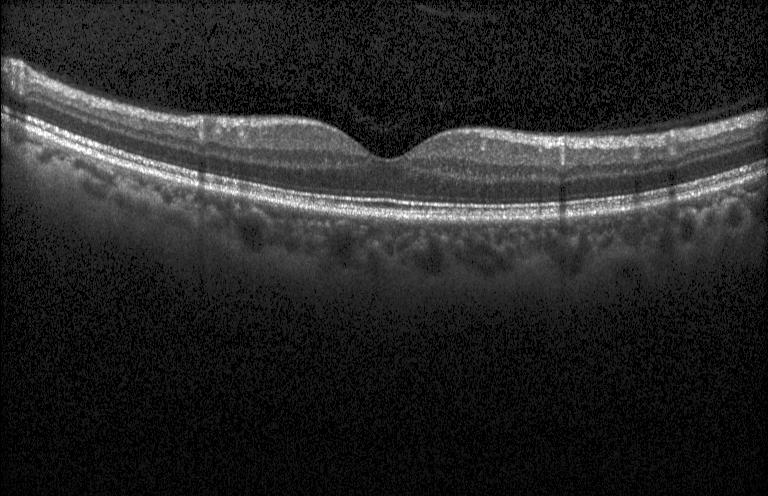 Instrument: Heidelberg Spectralis · optical coherence tomography B-scan — Diagnosis: neither choroidal neovascularization, diabetic macular edema, nor drusen.